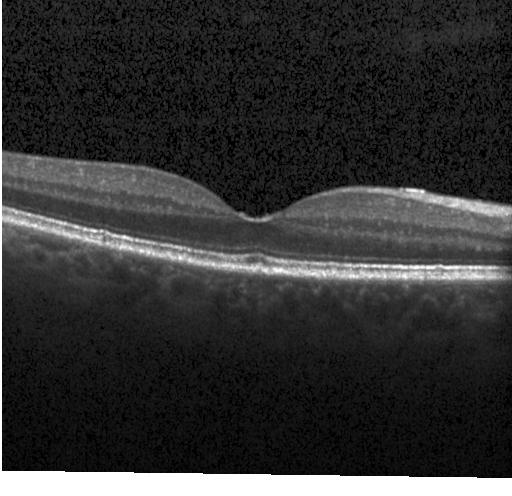
Spectral-domain OCT · optical coherence tomography B-scan · Heidelberg Spectralis · through the macula
No choroidal neovascularization, no diabetic macular edema, and no drusen.